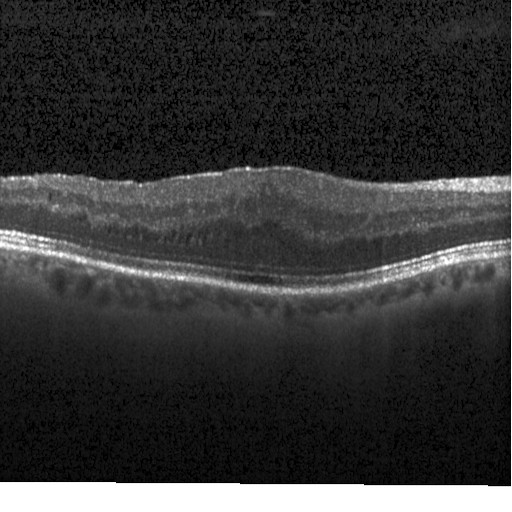
Impression: diabetic macular edema (DME).